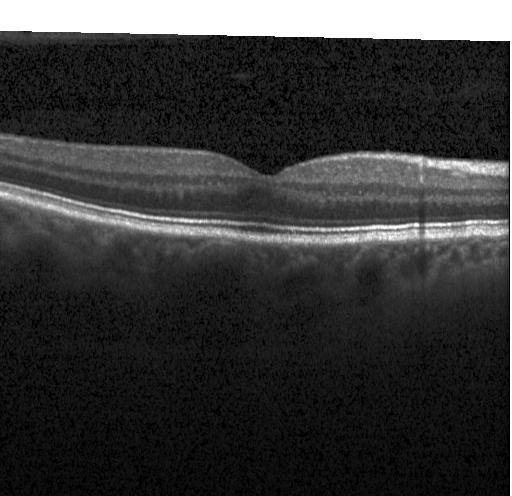

Heidelberg Spectralis · retinal OCT cross-section.
Impression: neither choroidal neovascularization, diabetic macular edema, nor drusen.